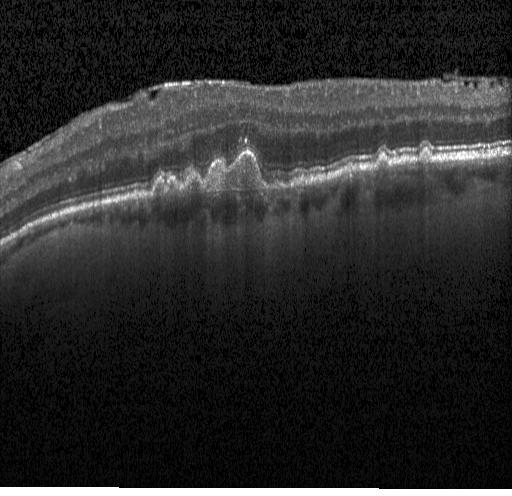

Finding: multiple drusen.